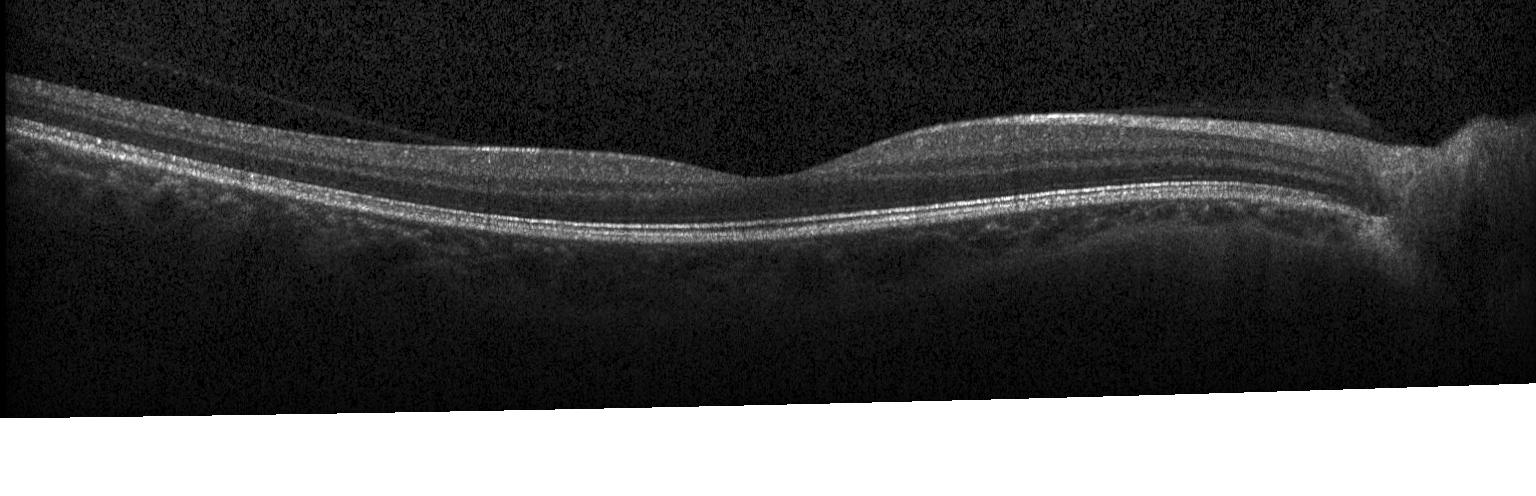
OCT line scan, Heidelberg Spectralis, horizontal scan through the fovea.
Assessment: no choroidal neovascularization, diabetic macular edema, or drusen.